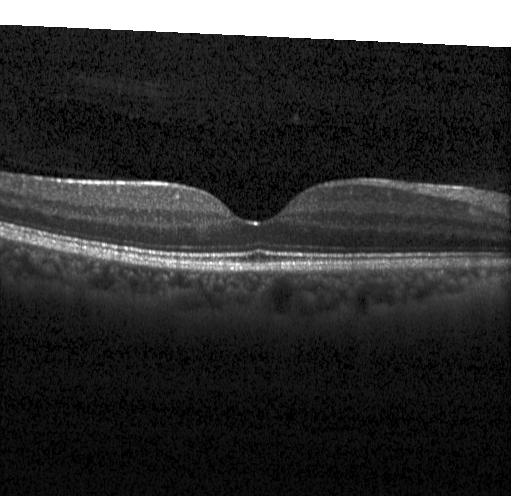 OCT B-scan.
Impression: neither choroidal neovascularization, diabetic macular edema, nor drusen.